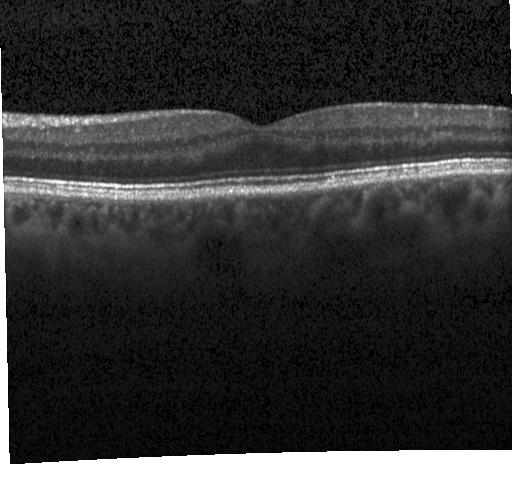

Diagnosis: neither CNV, DME, nor drusen.